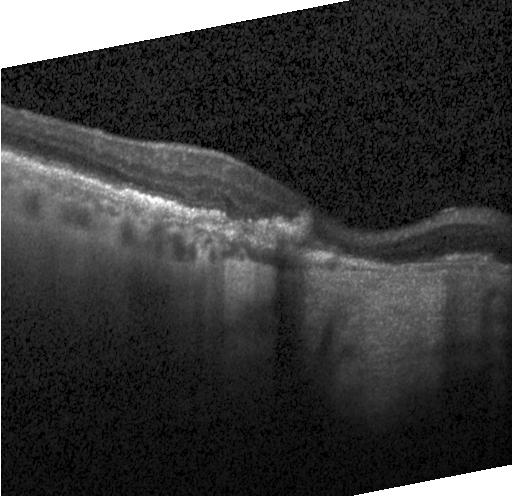

Acquired on a Heidelberg Spectralis. Fovea-centered. Optical coherence tomography B-scan. Spectral-domain OCT.
Diagnosis: choroidal neovascularization (CNV).